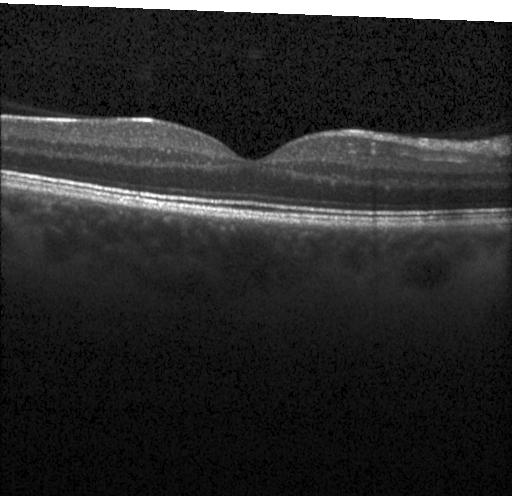

Macular scan; acquired on a Heidelberg Spectralis; OCT B-scan. Dx: no choroidal neovascularization, diabetic macular edema, or drusen.